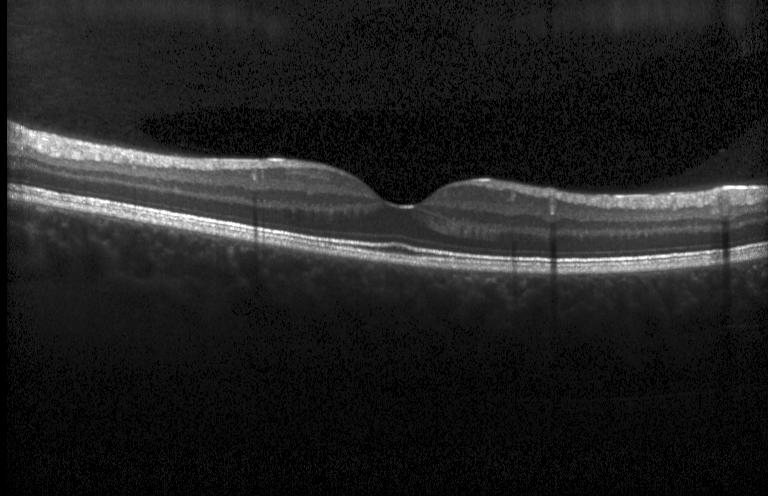

Dx: no evidence of CNV, DME, or drusen.